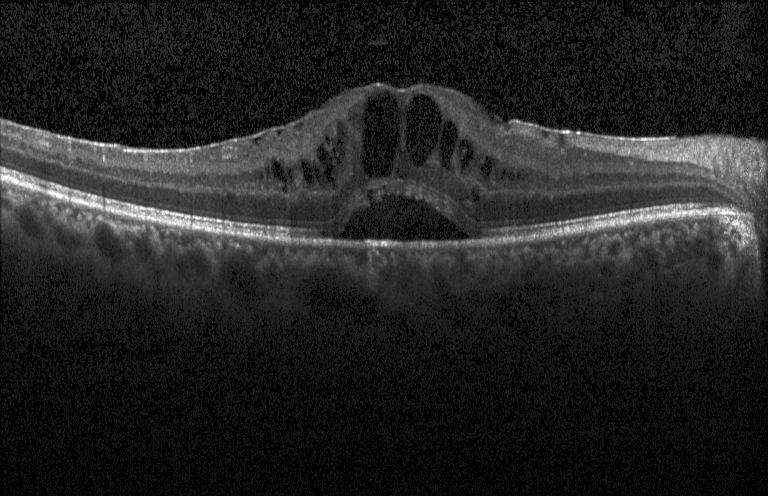
Dx: DME.